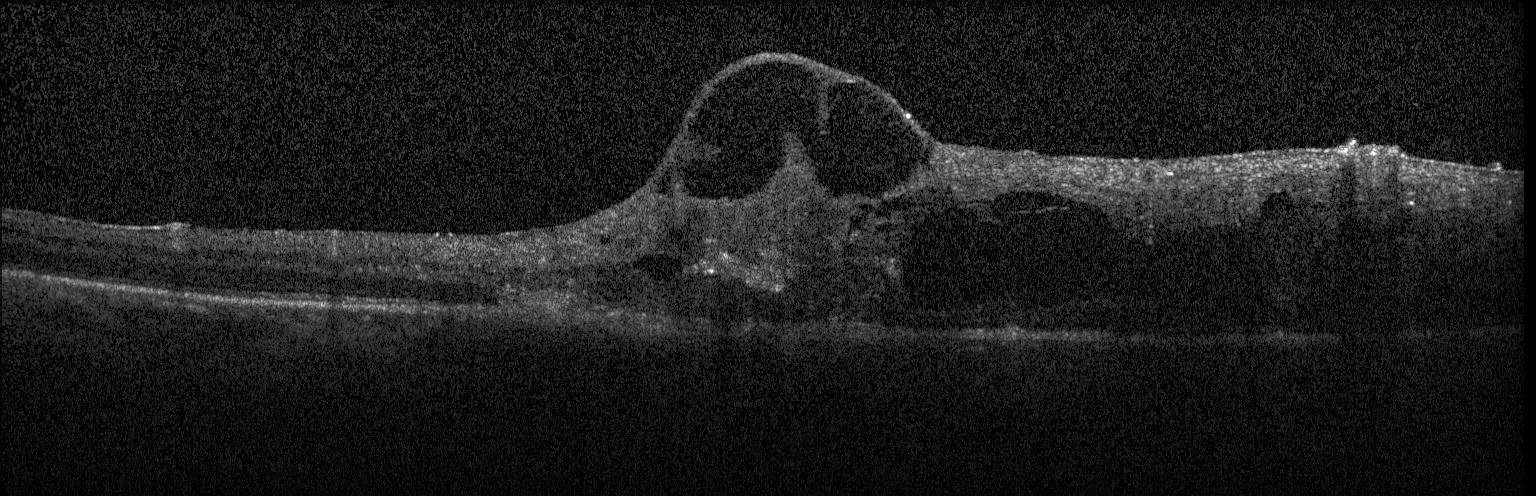
Assessment: a choroidal neovascular membrane.